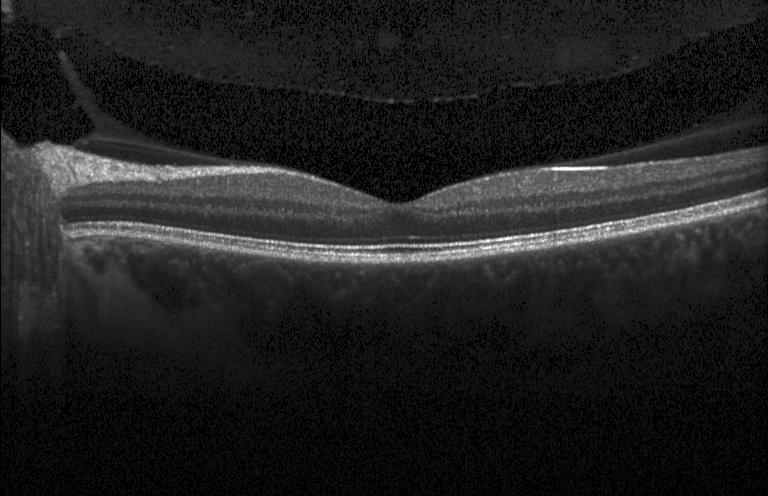

Spectral-domain optical coherence tomography · OCT line scan — Assessment: no evidence of CNV, DME, or drusen.